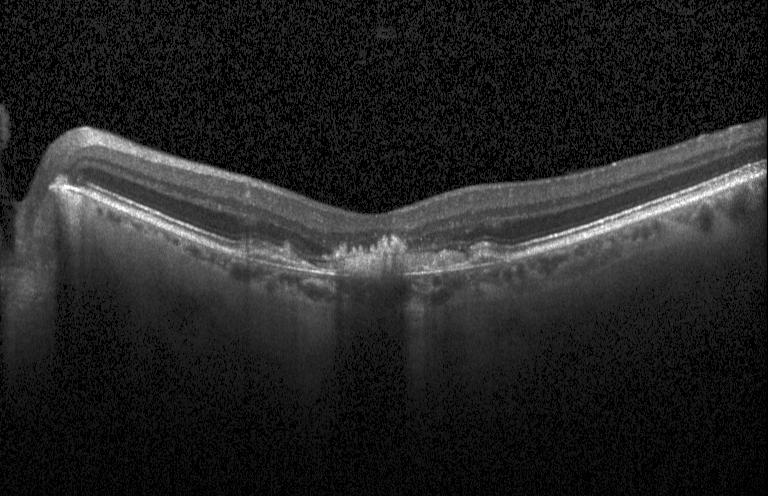

Instrument: Heidelberg Spectralis, spectral-domain optical coherence tomography, OCT B-scan
Diagnosis: CNV.